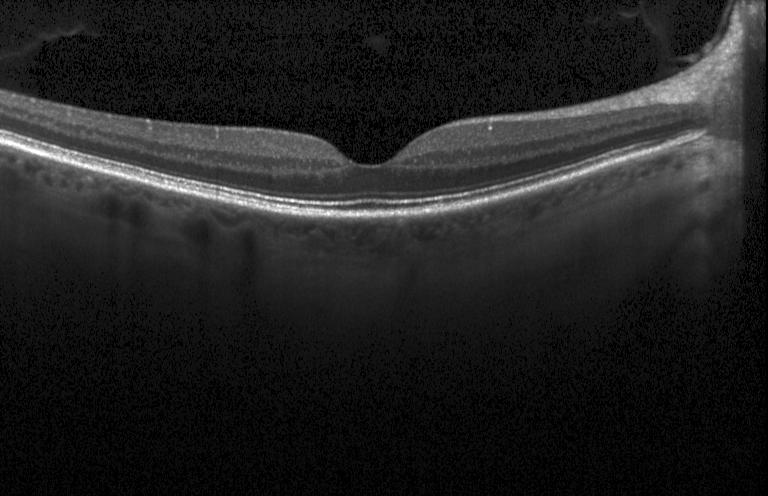

Retinal OCT cross-section showing no choroidal neovascularization, diabetic macular edema, or drusen.